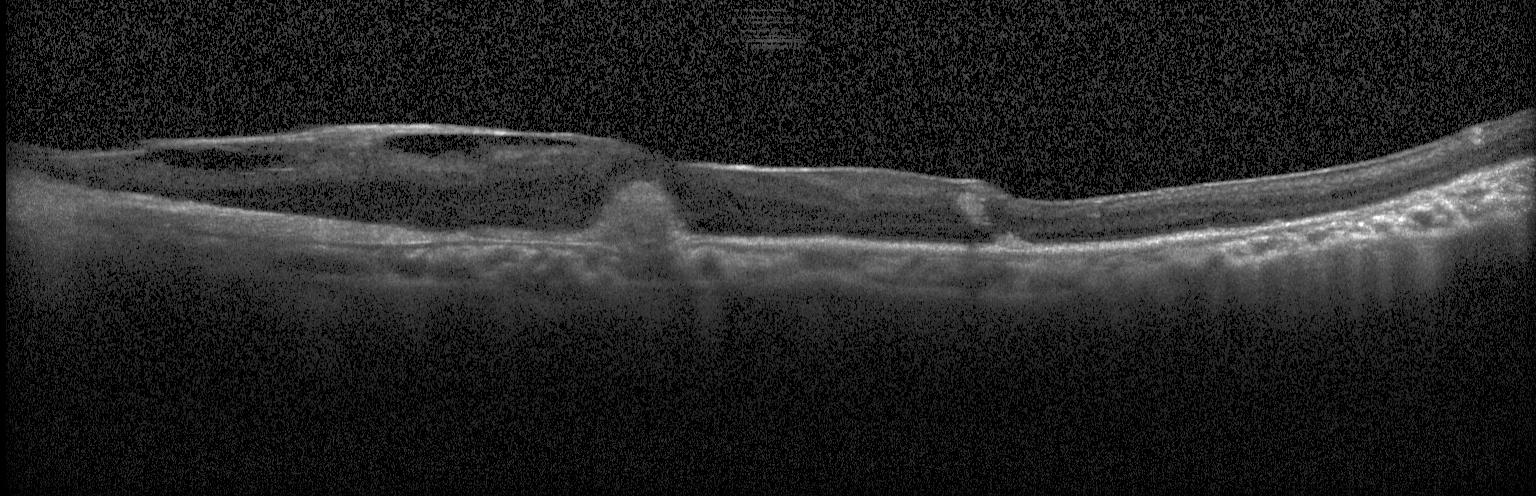
OCT B-scan — Impression: a choroidal neovascular membrane.